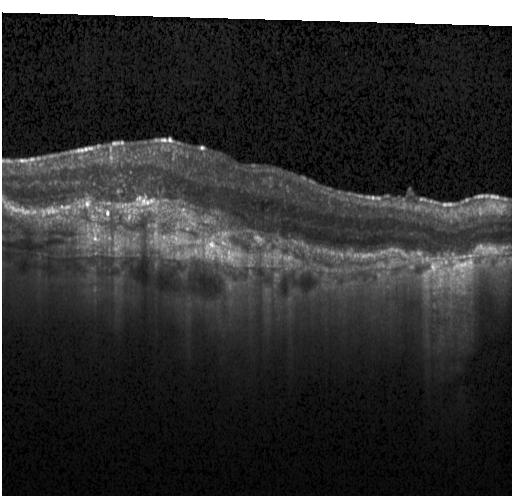 OCT B-scan.
Finding: choroidal neovascularization (CNV).